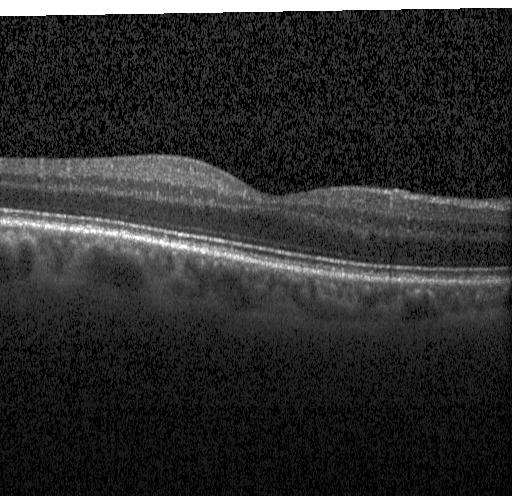

Acquired on a Heidelberg Spectralis; optical coherence tomography scan; through the macula; SD-OCT
No evidence of CNV, DME, or drusen.